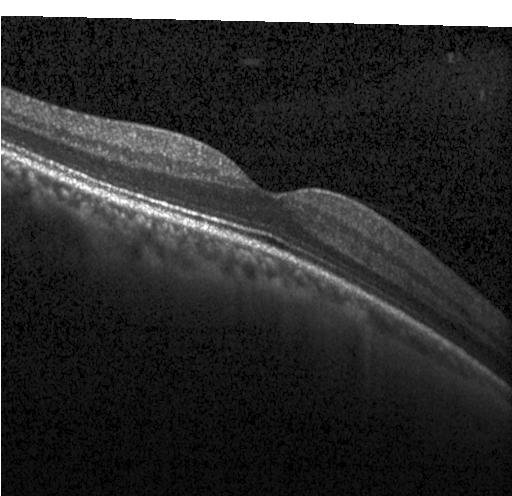 Retinal OCT B-scan. OCT finding: no choroidal neovascularization, no diabetic macular edema, and no drusen.